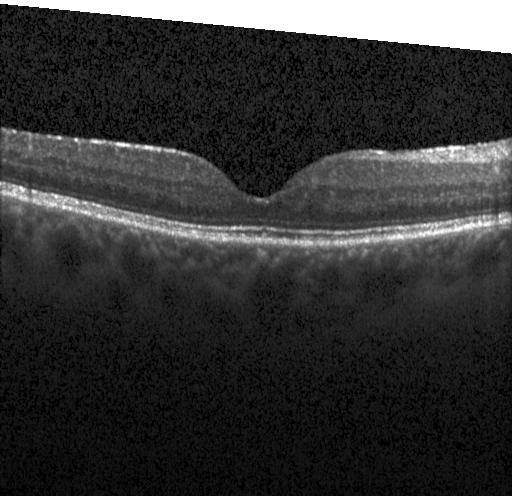

OCT B-scan — Assessment: no evidence of CNV, DME, or drusen.